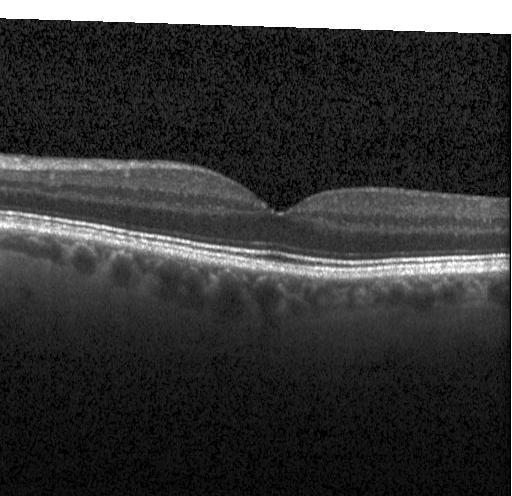

Centered on the fovea, retinal OCT cross-section, Heidelberg Spectralis OCT system. Diagnosis: no evidence of choroidal neovascularization, diabetic macular edema, or drusen.